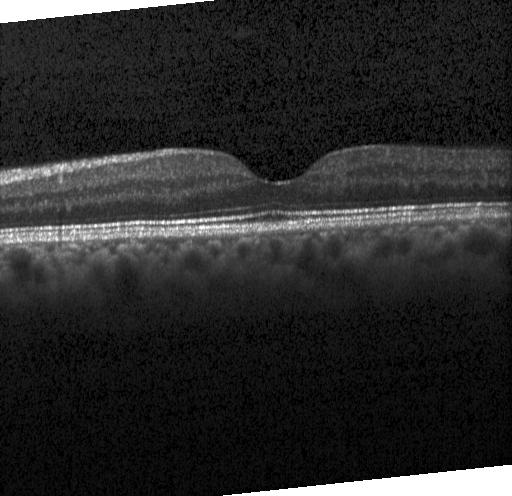
Diagnosis: no choroidal neovascularization, diabetic macular edema, or drusen.